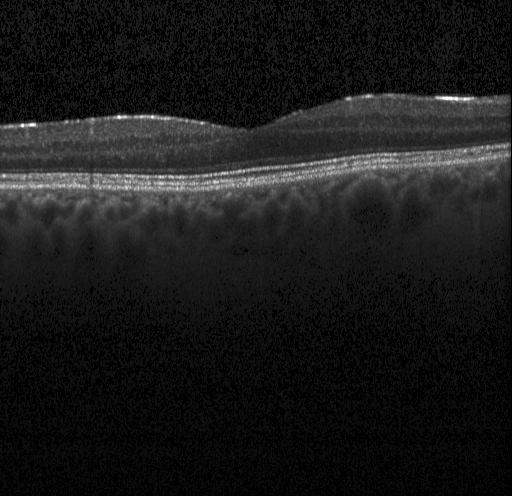

Heidelberg Spectralis; spectral-domain optical coherence tomography; fovea-centered; OCT line scan.
Finding: no CNV, no DME, and no drusen.